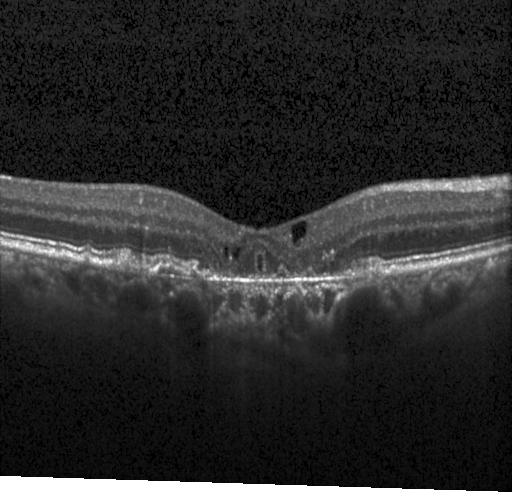 Retinal OCT cross-section; SD-OCT; fovea-centered; acquired on a Heidelberg Spectralis.
Diagnosis: choroidal neovascularization (CNV).